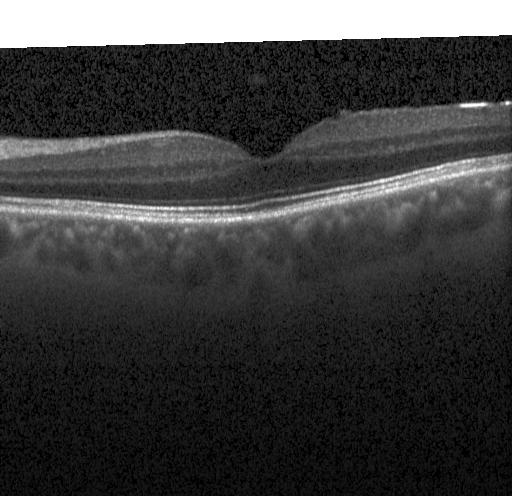
This B-scan demonstrates no evidence of CNV, DME, or drusen.